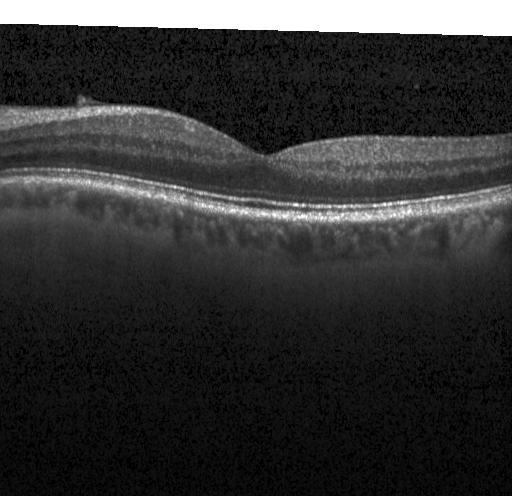 Retinal OCT cross-section showing neither choroidal neovascularization, diabetic macular edema, nor drusen.